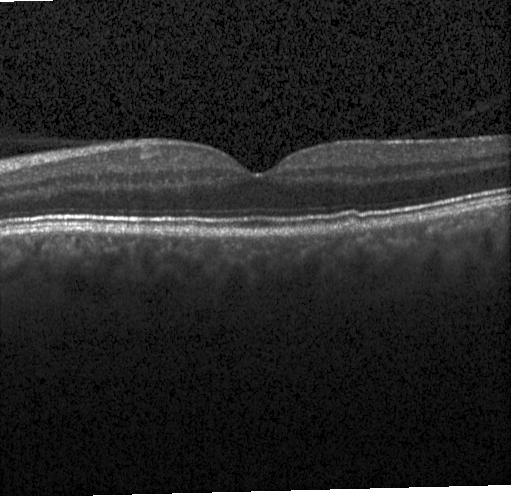
Diagnosis: sub-RPE drusenoid deposits.